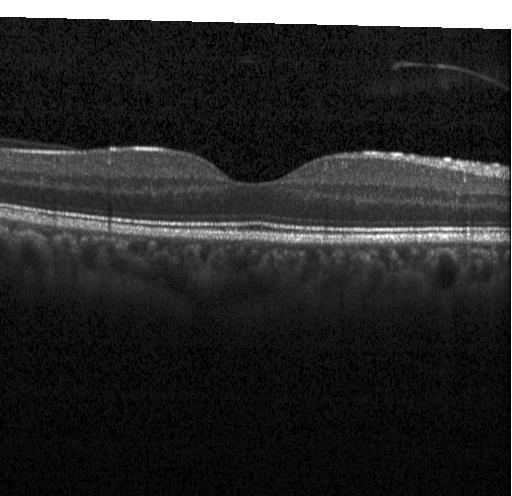
Diagnosis: no evidence of choroidal neovascularization, diabetic macular edema, or drusen.